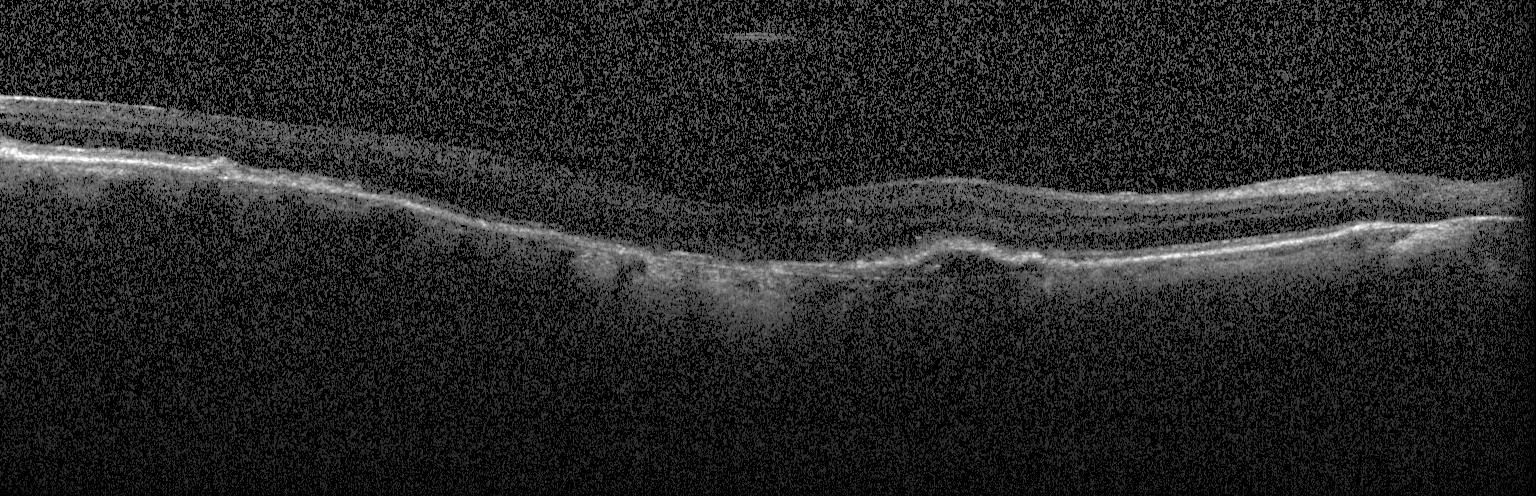
Macular OCT demonstrating choroidal neovascularization.